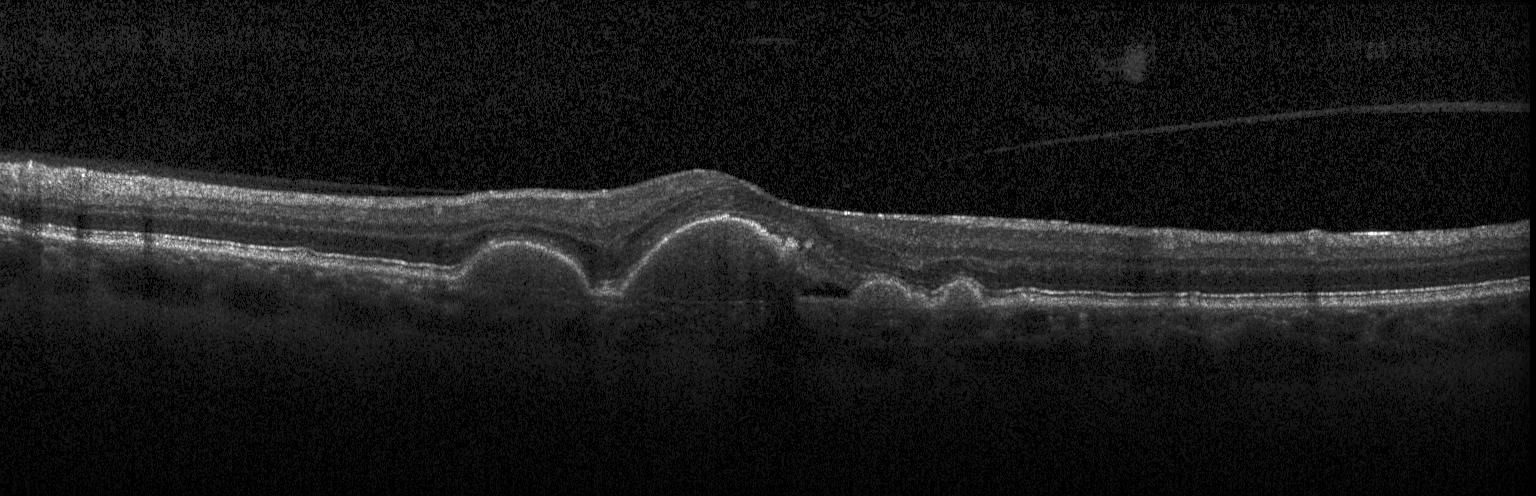
Optical coherence tomography scan, spectral-domain optical coherence tomography, macular scan, instrument: Heidelberg Spectralis. Assessment: choroidal neovascularization.